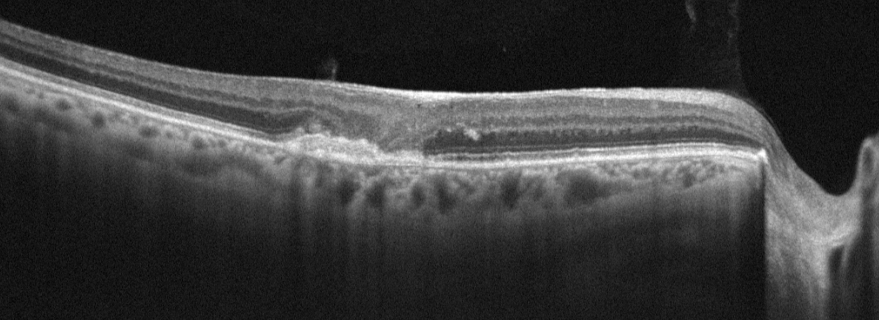
Retinal OCT B-scan. The scan shows AMD.